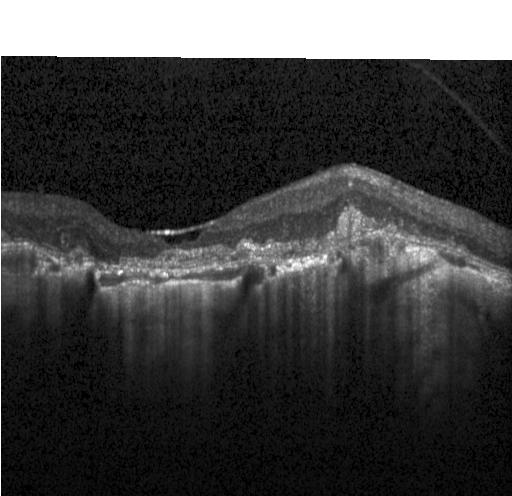 OCT scan showing choroidal neovascularization.